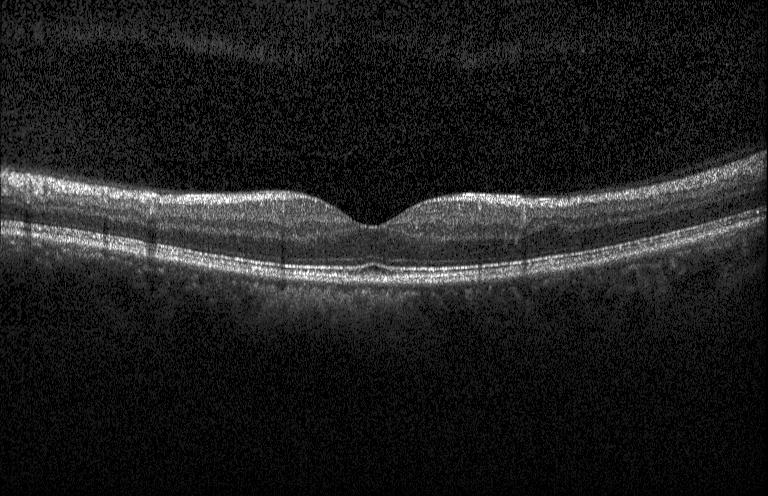 This B-scan demonstrates no choroidal neovascularization, no diabetic macular edema, and no drusen.